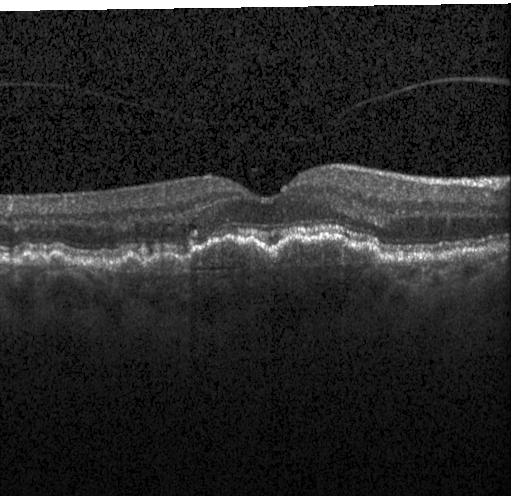
Spectral-domain OCT · instrument: Heidelberg Spectralis · through the macula · retinal OCT cross-section.
Impression: a choroidal neovascular membrane.